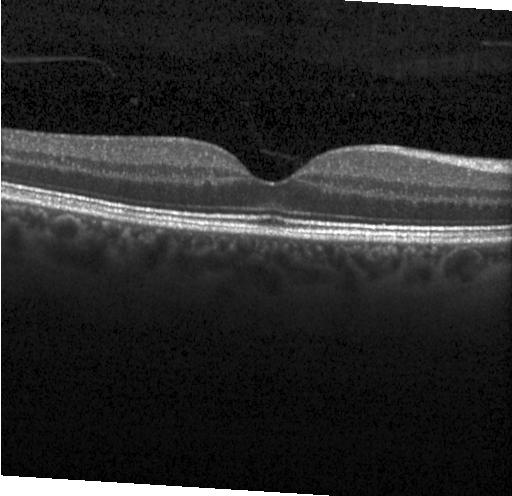 Through the macula. SD-OCT. Retinal OCT B-scan — Dx: no evidence of choroidal neovascularization, diabetic macular edema, or drusen.